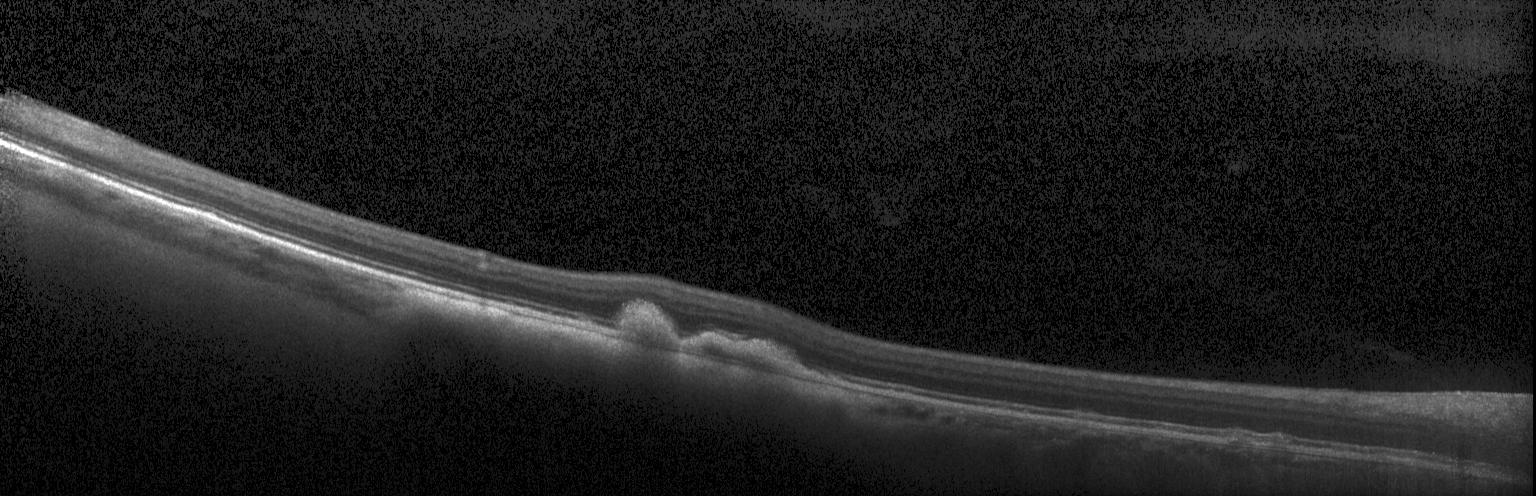 Spectral-domain OCT B-scan: CNV.